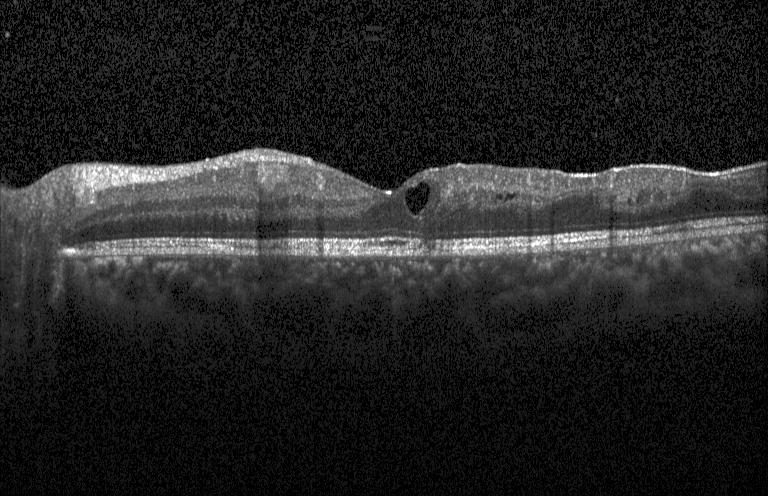 Heidelberg Spectralis, horizontal scan through the fovea, SD-OCT, retinal OCT cross-section
Finding: diabetic macular edema.